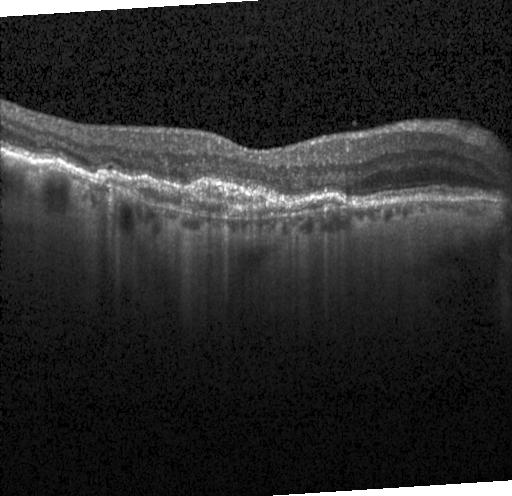

Finding: a choroidal neovascular membrane.